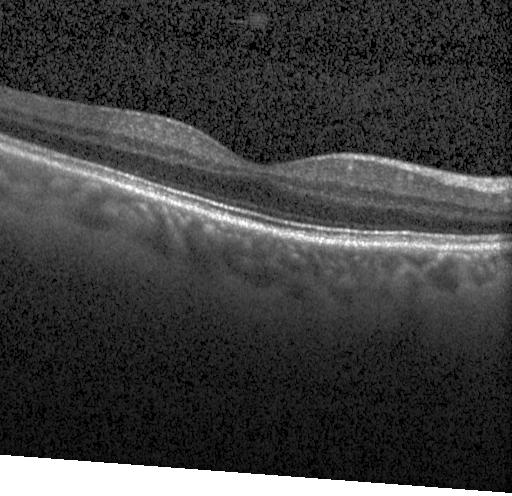
Heidelberg Spectralis, retinal OCT cross-section, macular scan. Impression: no evidence of CNV, DME, or drusen.